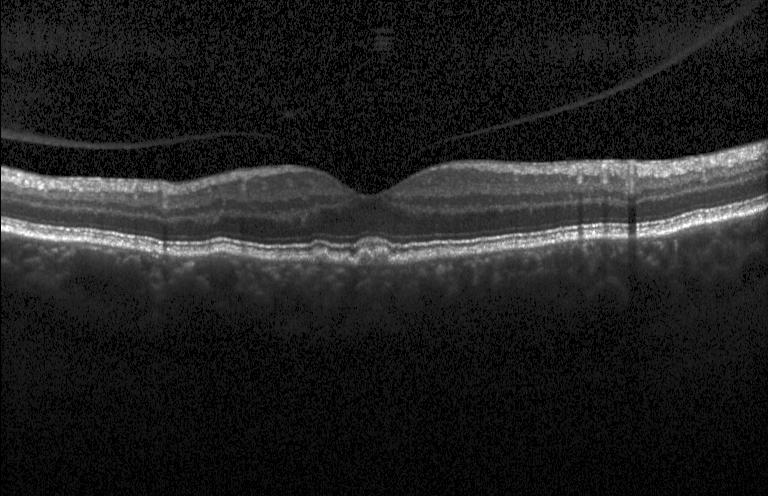

Impression: multiple drusen.